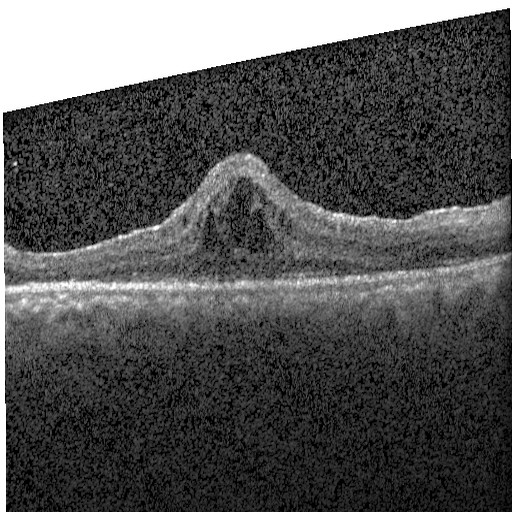

Dx: diabetic macular edema.